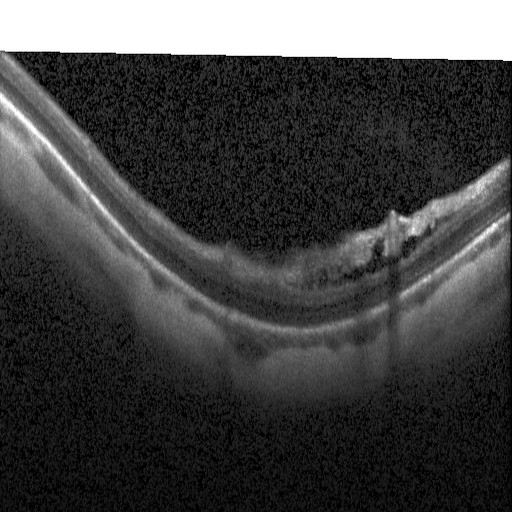 Acquired on a Heidelberg Spectralis. Optical coherence tomography scan — Dx: diabetic macular edema (DME).